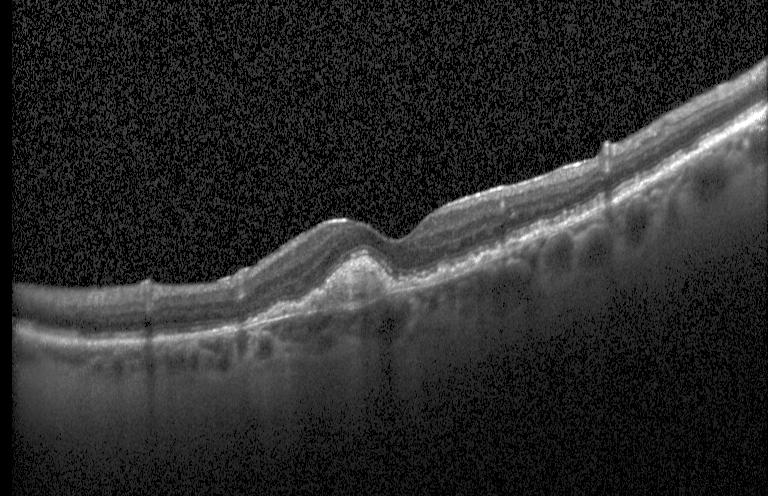 Dx: CNV.